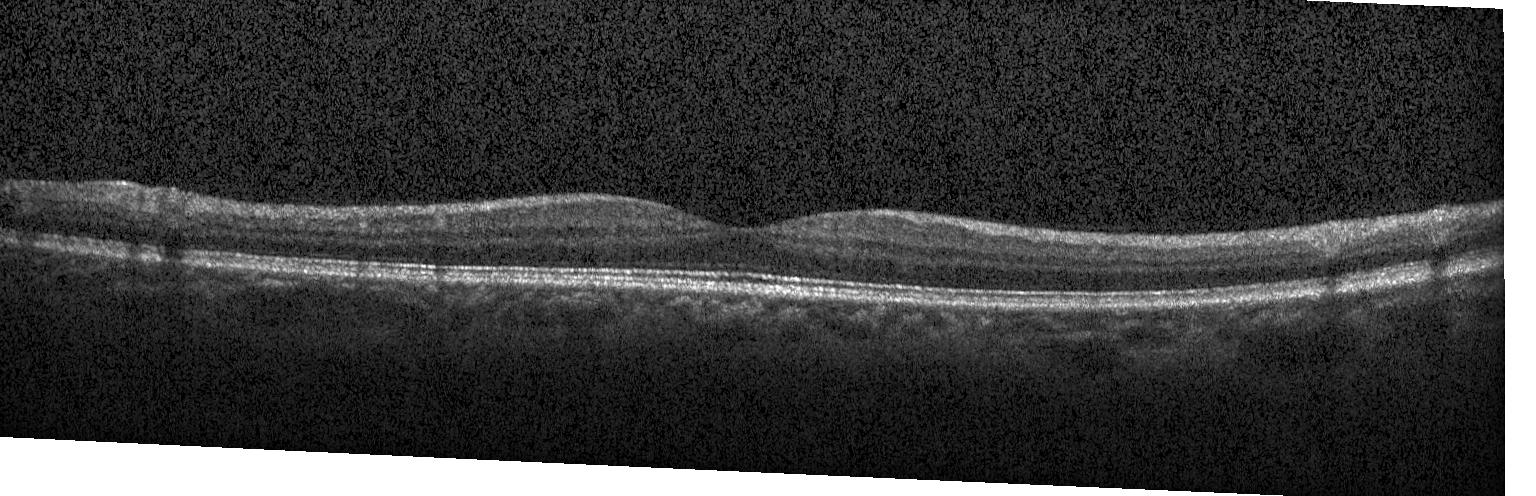 Centered on the fovea · OCT line scan · SD-OCT · Heidelberg Spectralis — Diagnosis: no evidence of CNV, DME, or drusen.